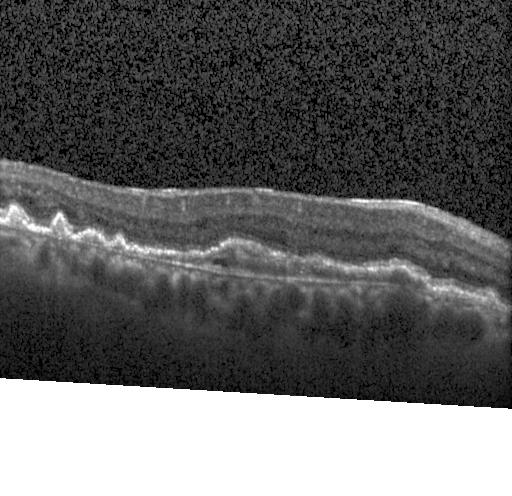

Optical coherence tomography B-scan · acquired on a Heidelberg Spectralis — Finding: a choroidal neovascular membrane.